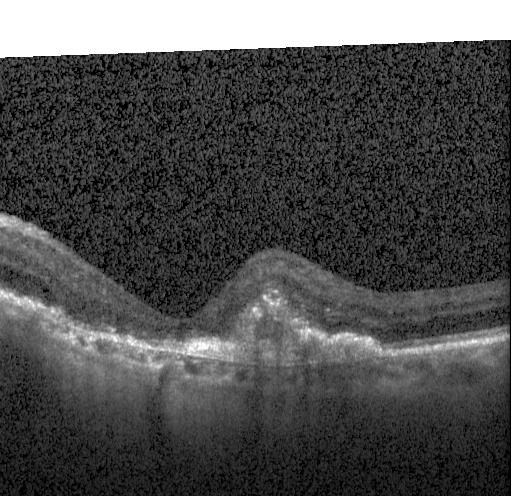

Retinal OCT cross-section. Spectral-domain optical coherence tomography. Dx: choroidal neovascularization (CNV).